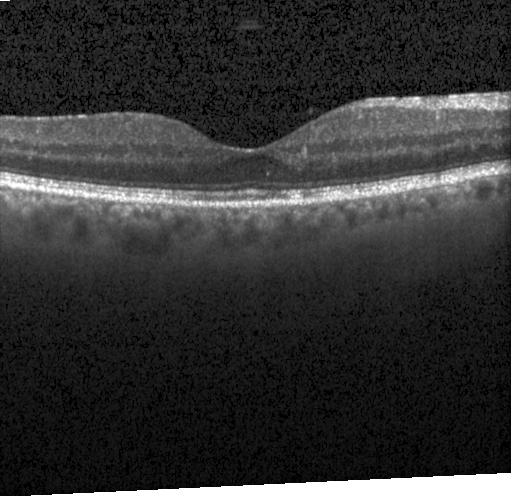

Retinal OCT B-scan · instrument: Heidelberg Spectralis.
Diagnosis: no choroidal neovascularization, no diabetic macular edema, and no drusen.